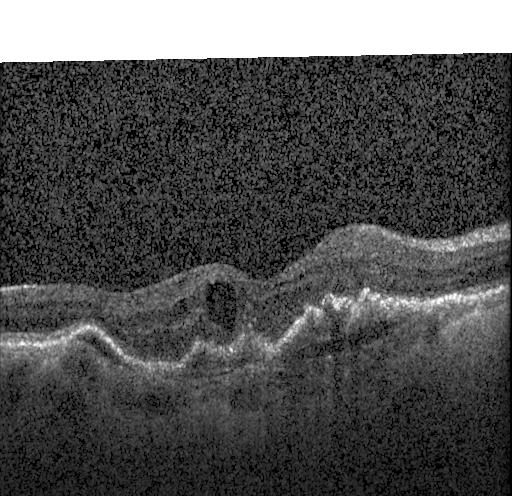
Impression: a choroidal neovascular membrane.